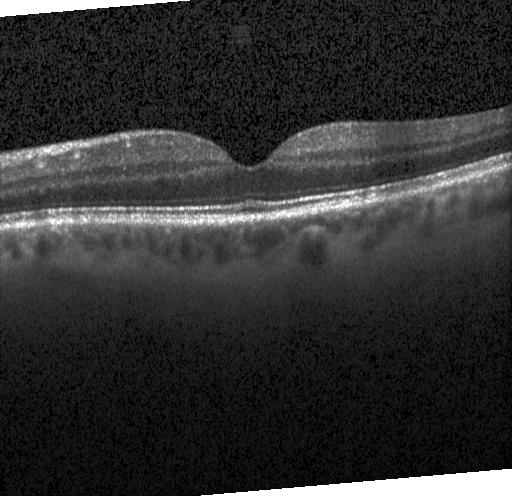
Acquired on a Heidelberg Spectralis; SD-OCT; retinal OCT cross-section; through the macula
Impression: no choroidal neovascularization, no diabetic macular edema, and no drusen.